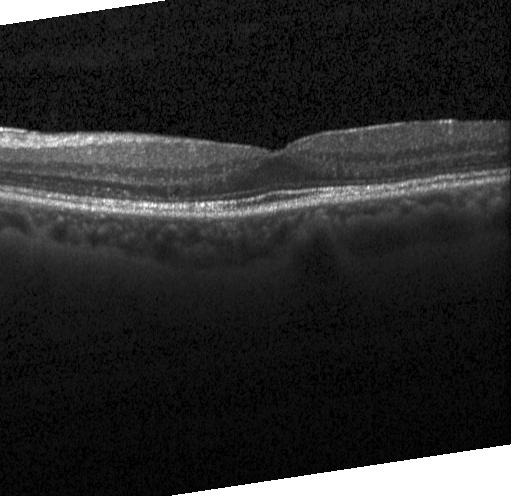

Finding: neither choroidal neovascularization, diabetic macular edema, nor drusen.